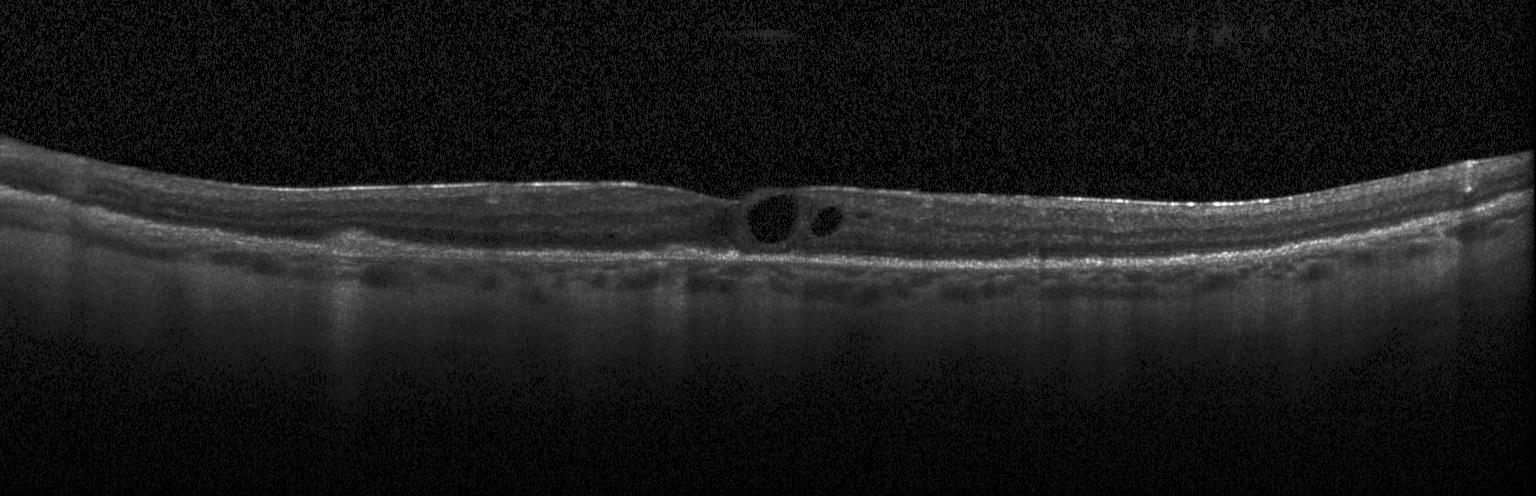 Optical coherence tomography scan. Impression: a choroidal neovascular membrane.